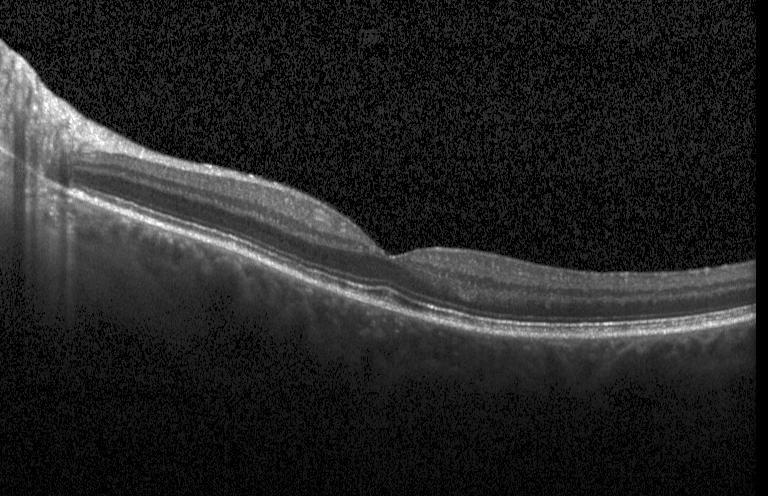
Dx: no choroidal neovascularization, no diabetic macular edema, and no drusen.